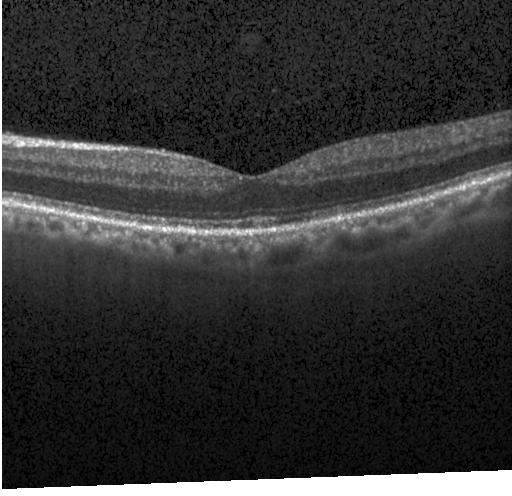 Instrument: Heidelberg Spectralis; OCT B-scan; spectral-domain OCT; horizontal scan through the fovea. Macular OCT: no evidence of choroidal neovascularization, diabetic macular edema, or drusen.